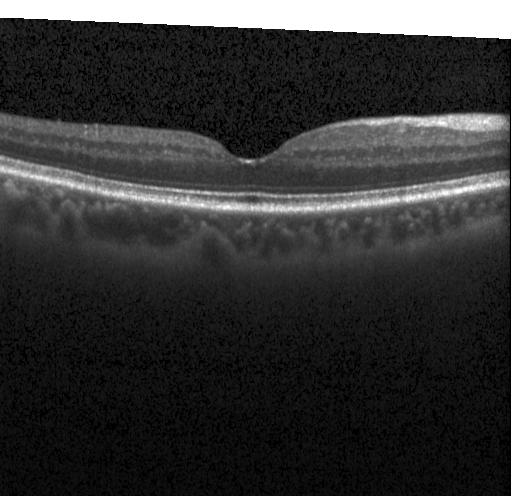
Diagnosis: neither choroidal neovascularization, diabetic macular edema, nor drusen.